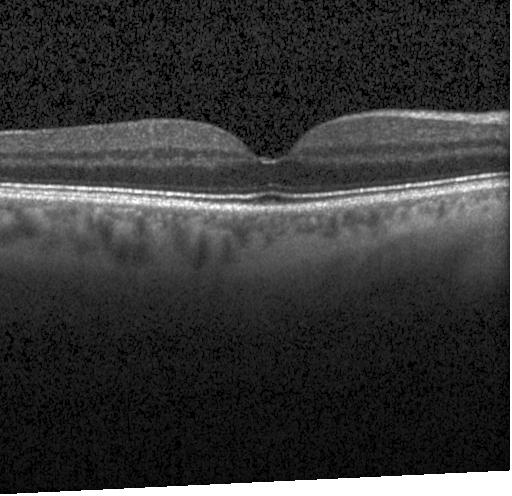
The scan shows no choroidal neovascularization, no diabetic macular edema, and no drusen.